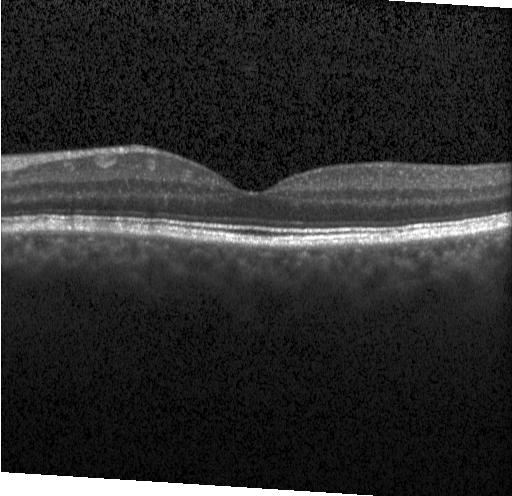

Optical coherence tomography scan · spectral-domain OCT
No choroidal neovascularization, no diabetic macular edema, and no drusen.